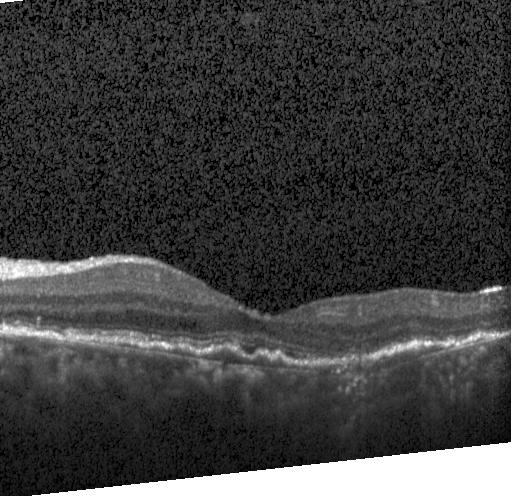
OCT line scan
Diagnosis: choroidal neovascularization (CNV).